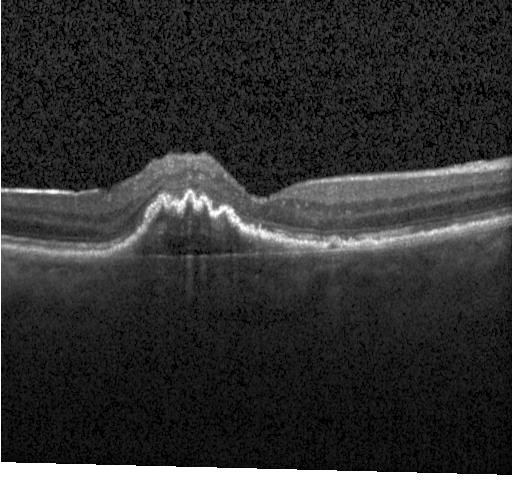
Assessment: a choroidal neovascular membrane.